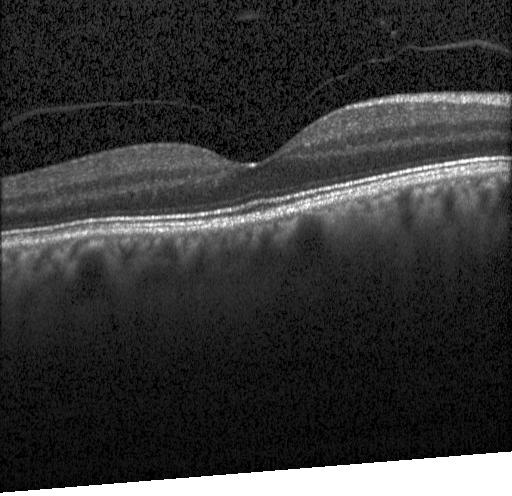 Assessment: no evidence of CNV, DME, or drusen.